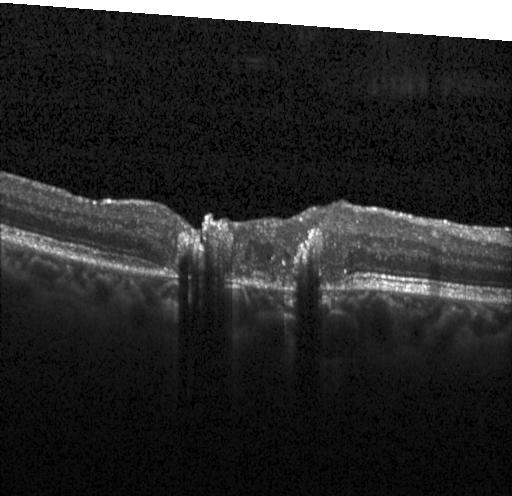 Spectral-domain OCT. Centered on the fovea. Optical coherence tomography B-scan. Heidelberg Spectralis OCT system. Assessment: a choroidal neovascular membrane.